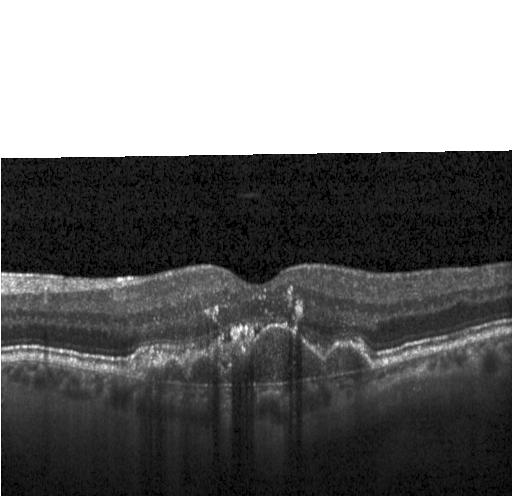
OCT finding: a choroidal neovascular membrane.